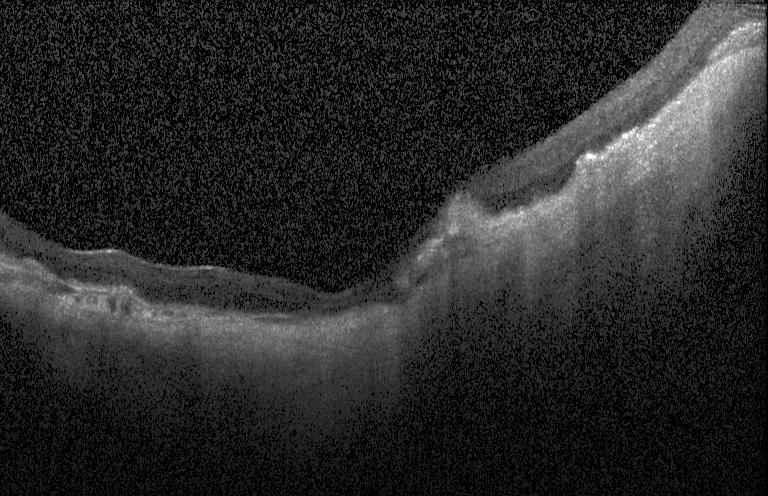
Retinal OCT cross-section.
Diagnosis: choroidal neovascularization (CNV).